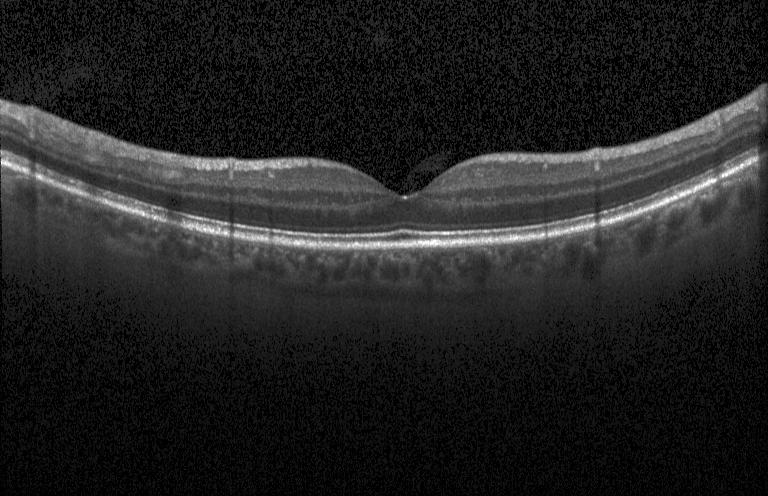

Heidelberg Spectralis OCT system. Retinal OCT cross-section. Fovea-centered
Diagnosis: no evidence of choroidal neovascularization, diabetic macular edema, or drusen.